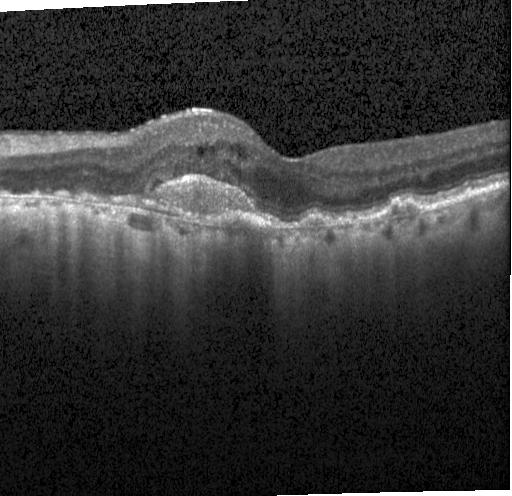
Assessment: a choroidal neovascular membrane.